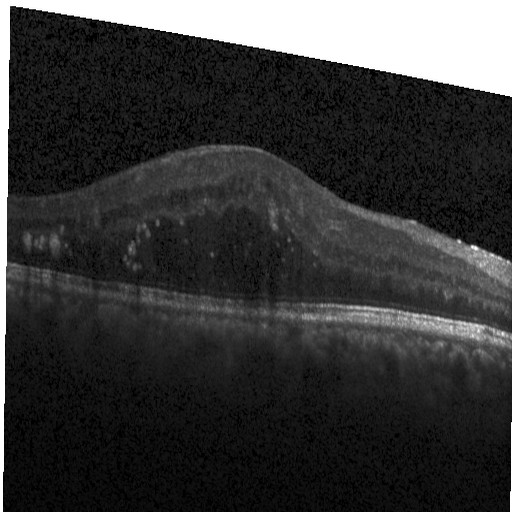 Instrument: Heidelberg Spectralis; macular scan; retinal OCT B-scan
Assessment: diabetic macular edema (DME).